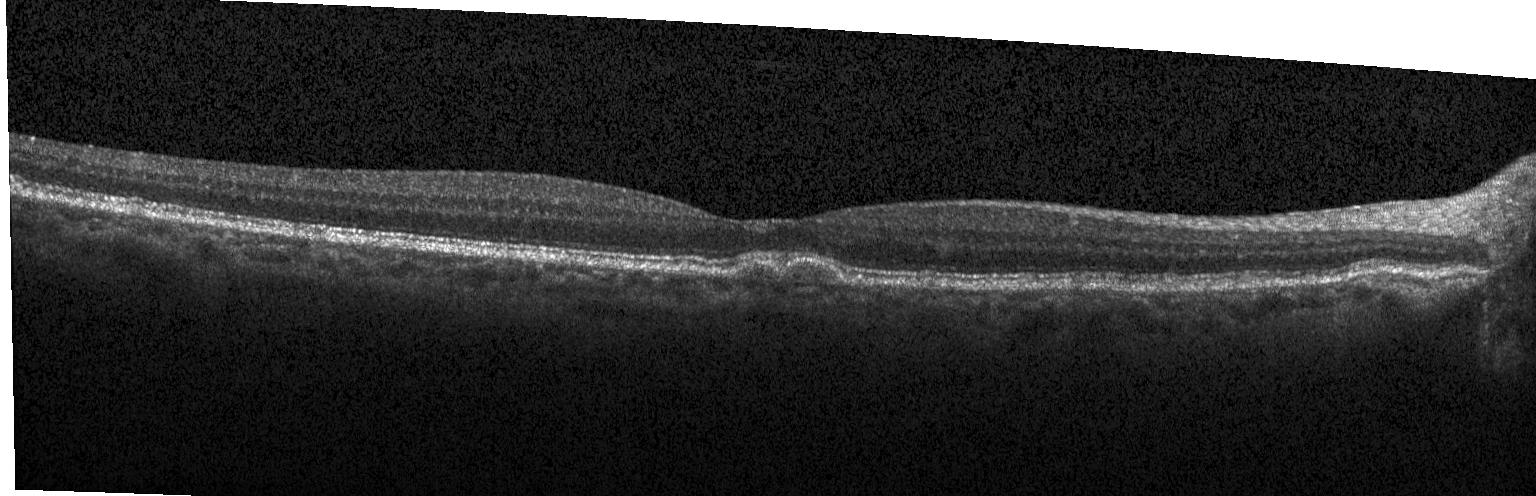
Retinal OCT cross-section — Impression: sub-RPE drusenoid deposits.